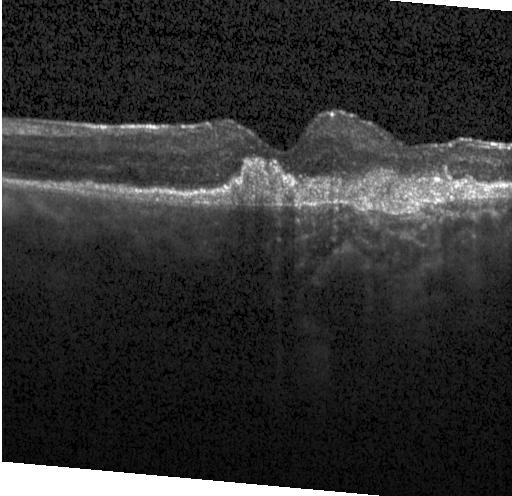

Retinal OCT B-scan · SD-OCT · centered on the fovea.
Impression: CNV.